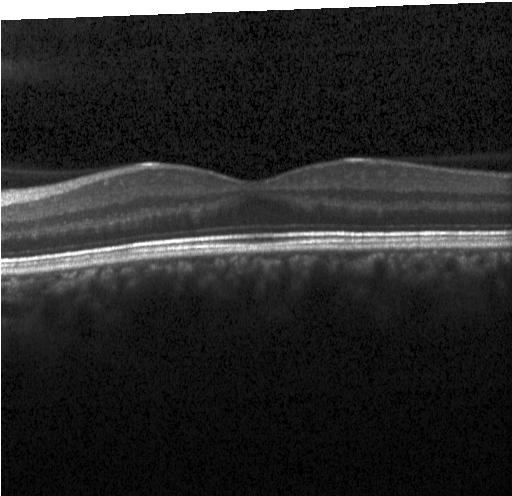 Optical coherence tomography B-scan. Instrument: Heidelberg Spectralis. Spectral-domain OCT. Macular scan — Macular OCT: no CNV, no DME, and no drusen.